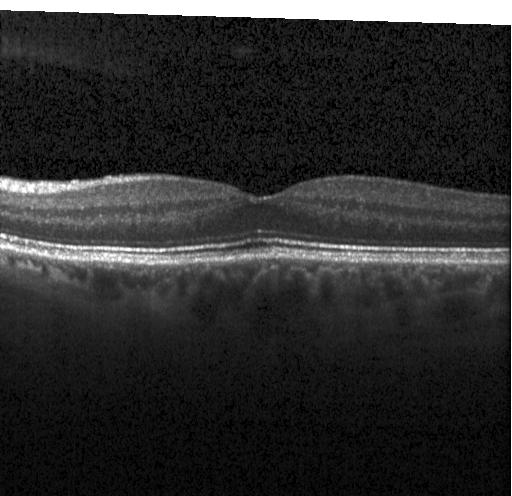
OCT B-scan — Dx: no choroidal neovascularization, no diabetic macular edema, and no drusen.